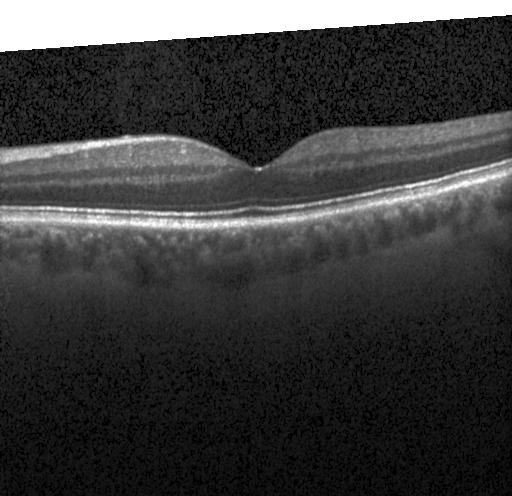 Dx: no evidence of choroidal neovascularization, diabetic macular edema, or drusen.